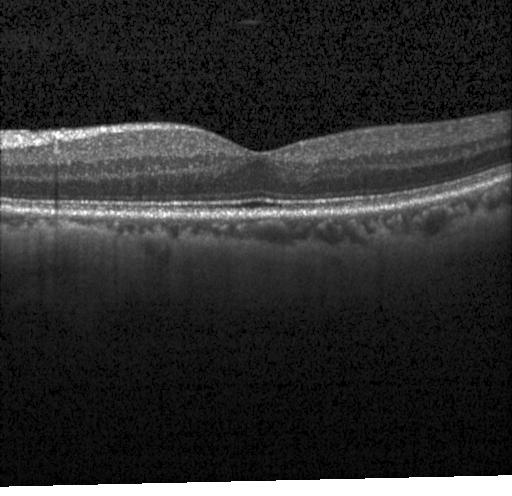

Spectral-domain optical coherence tomography; Heidelberg Spectralis OCT system; horizontal scan through the fovea; optical coherence tomography scan — This B-scan demonstrates no CNV, no DME, and no drusen.